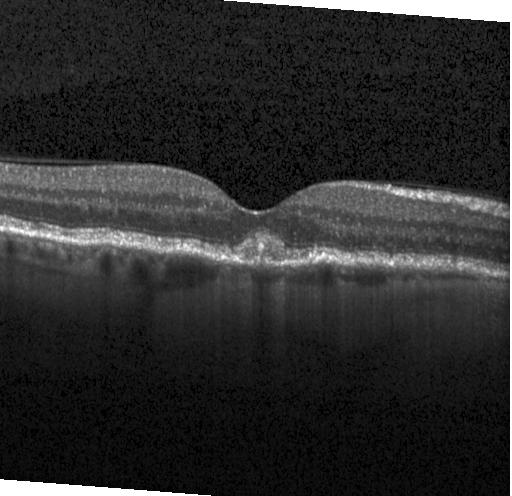 Finding: sub-RPE drusenoid deposits.